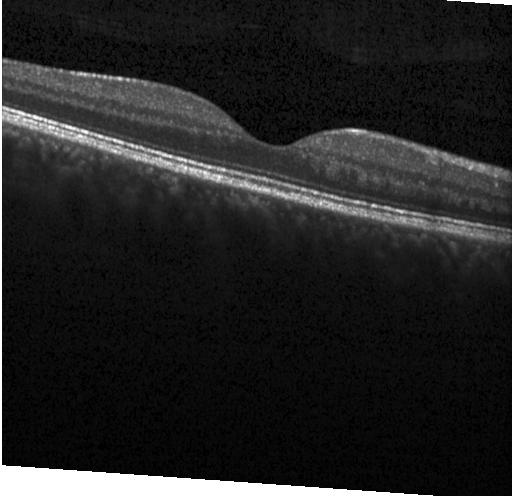
OCT finding: no choroidal neovascularization, no diabetic macular edema, and no drusen.